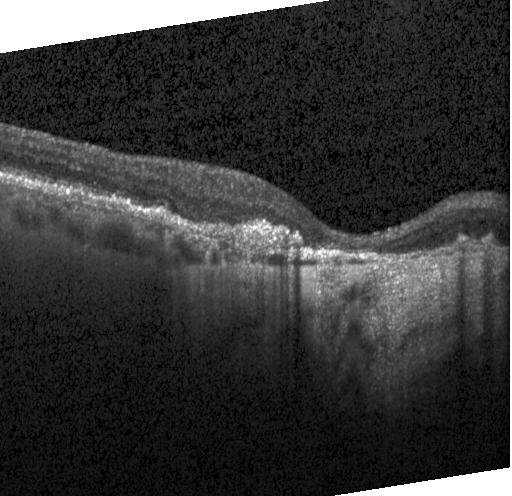 OCT B-scan; Heidelberg Spectralis; spectral-domain OCT; macular scan
A choroidal neovascular membrane.